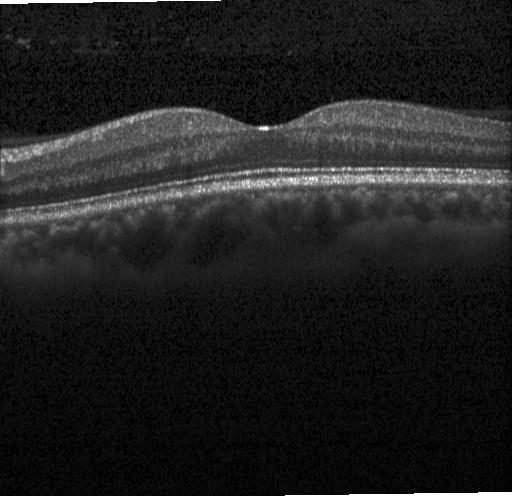

Optical coherence tomography B-scan — Dx: no choroidal neovascularization, no diabetic macular edema, and no drusen.